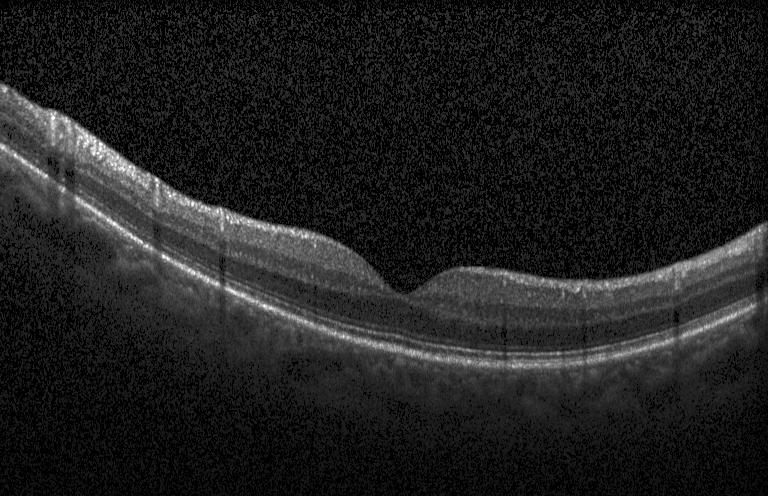 Finding: no CNV, no DME, and no drusen.